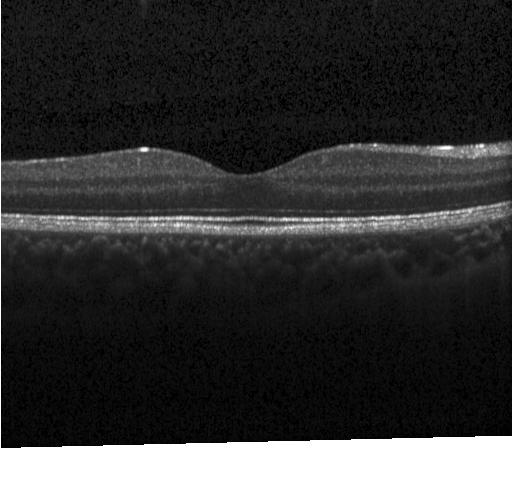
Spectral-domain optical coherence tomography. Optical coherence tomography scan.
No evidence of CNV, DME, or drusen.